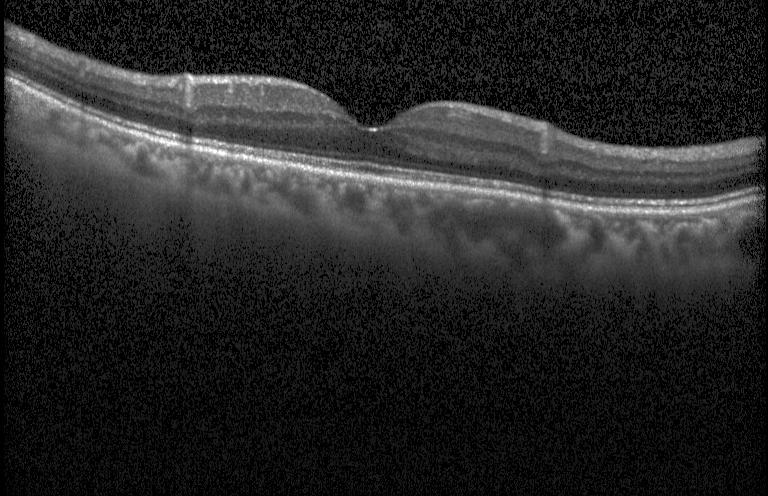 OCT line scan · through the macula · Heidelberg Spectralis OCT system · SD-OCT
Impression: neither choroidal neovascularization, diabetic macular edema, nor drusen.